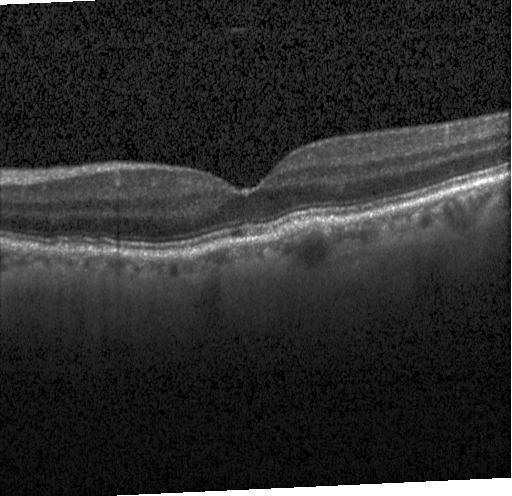

This B-scan demonstrates sub-RPE drusenoid deposits.